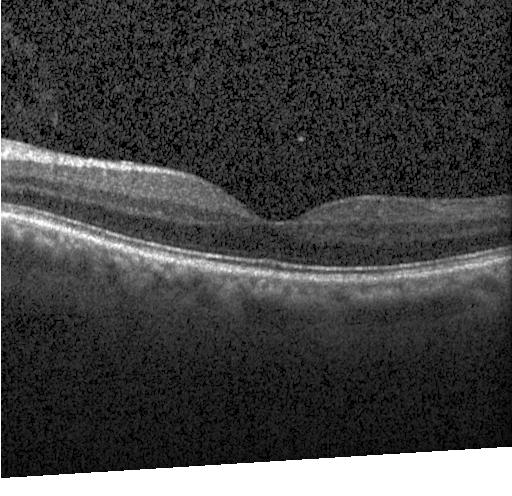

Finding: no evidence of choroidal neovascularization, diabetic macular edema, or drusen.